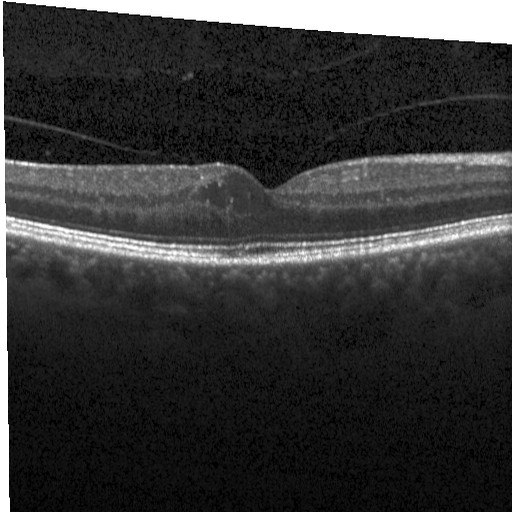
OCT B-scan. Impression: diabetic macular edema (DME).